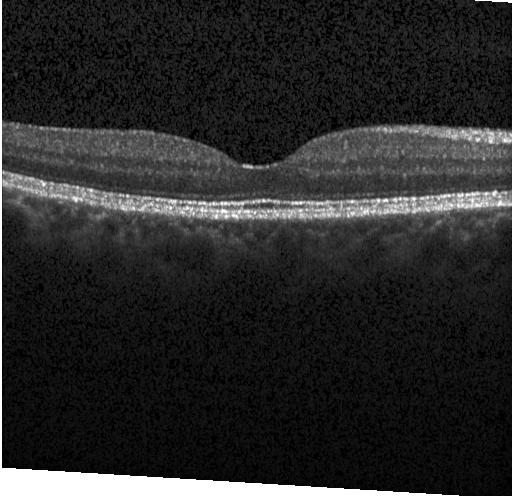
Retinal OCT B-scan · spectral-domain optical coherence tomography
This B-scan demonstrates no choroidal neovascularization, no diabetic macular edema, and no drusen.